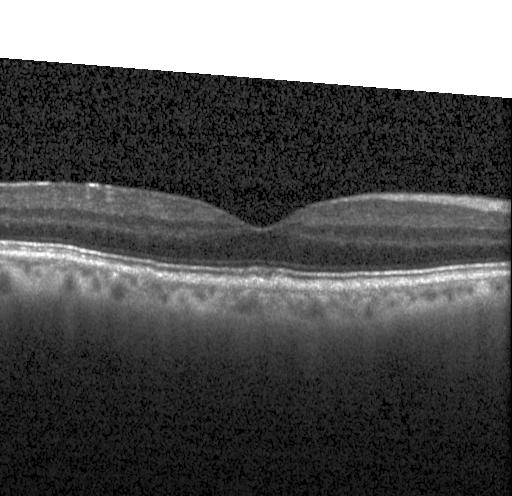 This B-scan demonstrates no evidence of choroidal neovascularization, diabetic macular edema, or drusen.